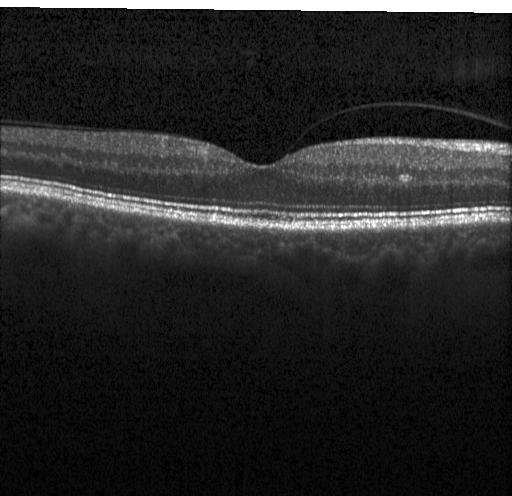
Retinal OCT B-scan. Spectral-domain OCT. Macular OCT: no choroidal neovascularization, no diabetic macular edema, and no drusen.